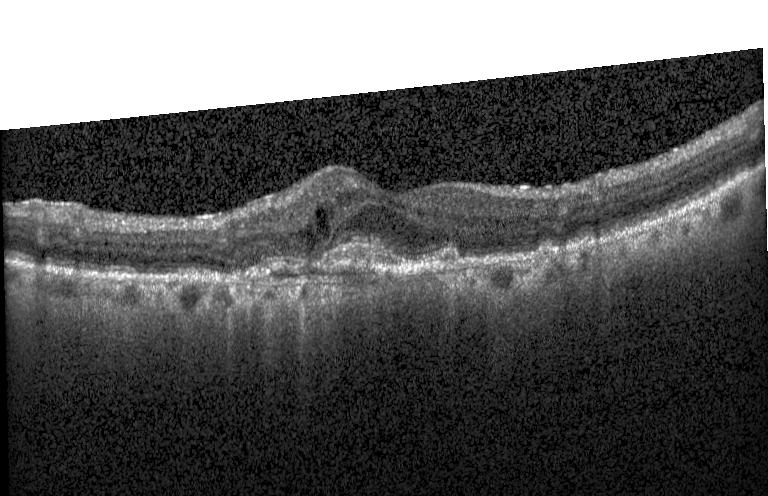

Macular OCT: a choroidal neovascular membrane.